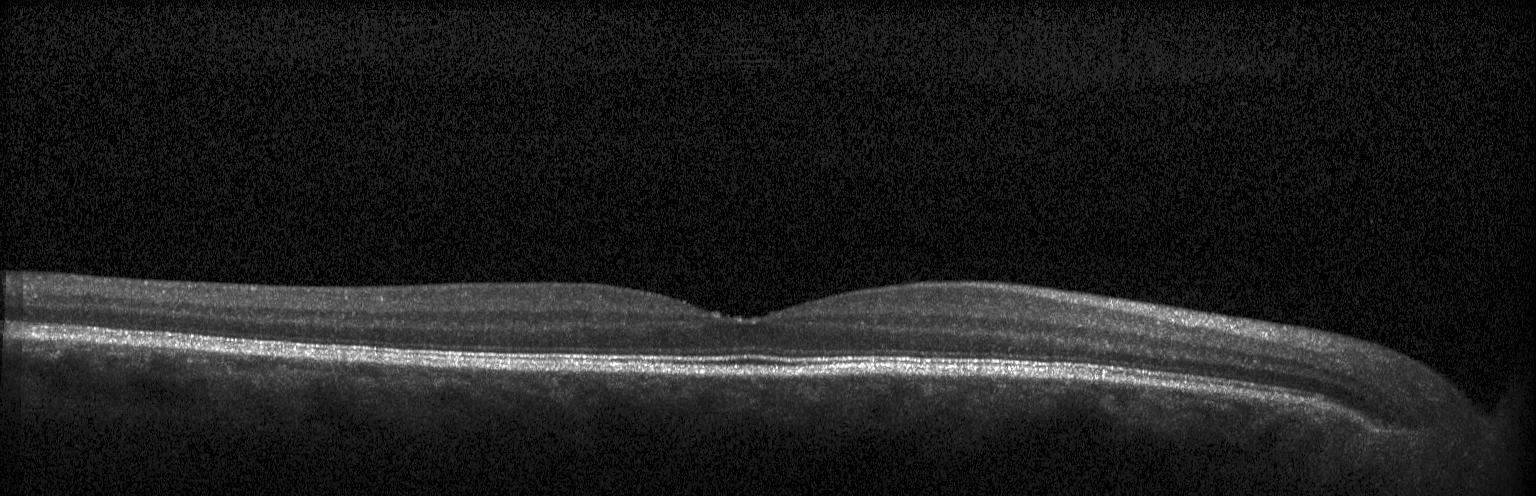
Optical coherence tomography scan
OCT finding: no choroidal neovascularization, diabetic macular edema, or drusen.